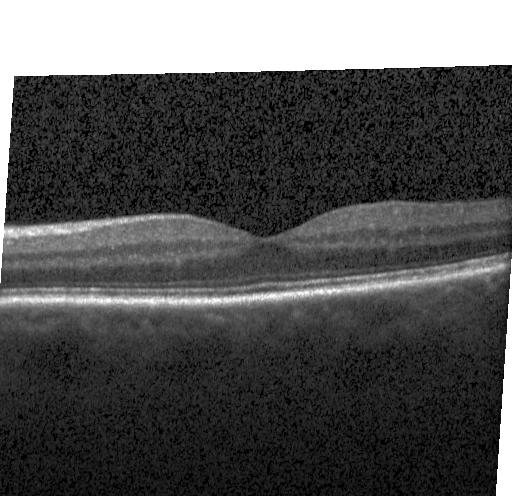 Heidelberg Spectralis OCT system. Horizontal scan through the fovea. Retinal OCT cross-section.
The scan shows no evidence of choroidal neovascularization, diabetic macular edema, or drusen.